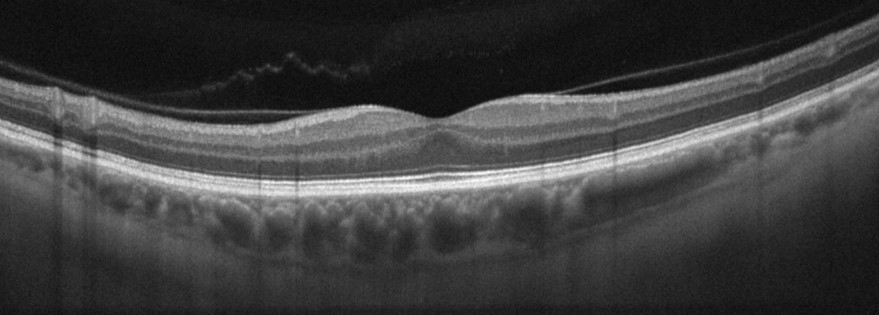 Macular scan, acquired on an Optovue Avanti RTVue XR, retinal OCT B-scan.
Assessment: absence of AMD, DME, ERM, RAO, RVO, and vitreomacular interface disease.